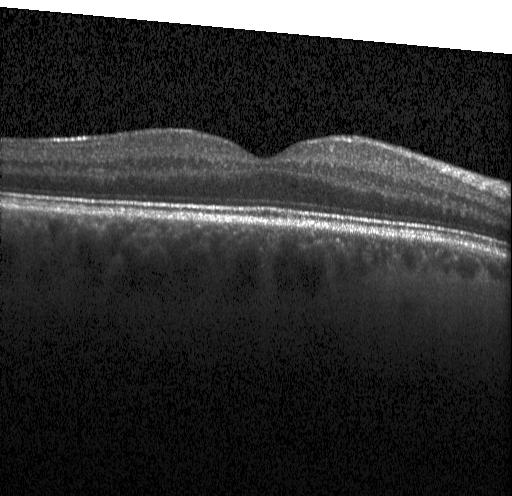

Retinal OCT cross-section · Heidelberg Spectralis OCT system · through the macula. Finding: no evidence of CNV, DME, or drusen.